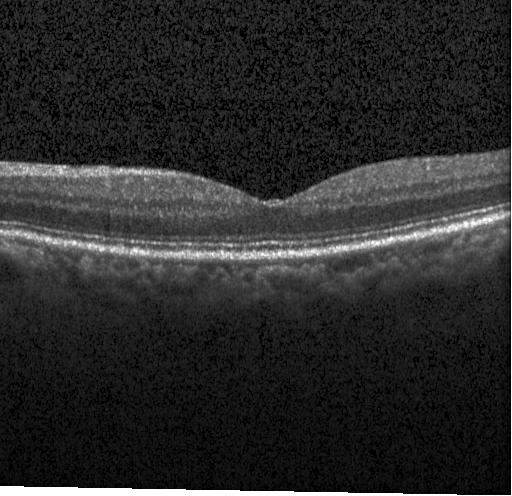
Macular OCT demonstrating no evidence of choroidal neovascularization, diabetic macular edema, or drusen.